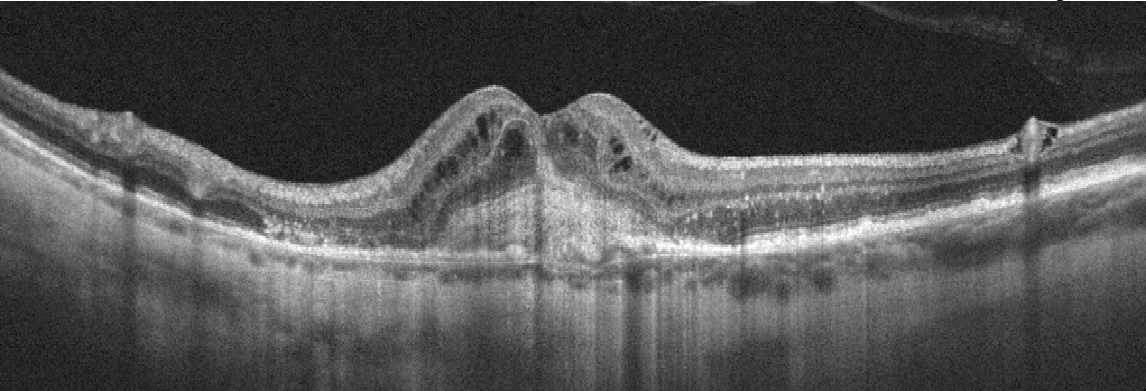
Optical coherence tomography B-scan · Optovue Avanti RTVue XR — OCT finding: age-related macular degeneration.